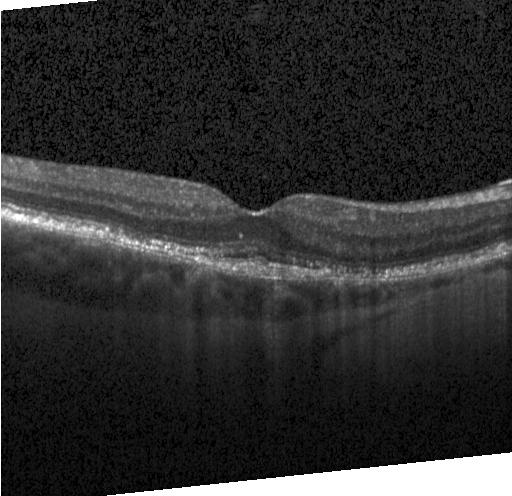 Macular OCT: a choroidal neovascular membrane.